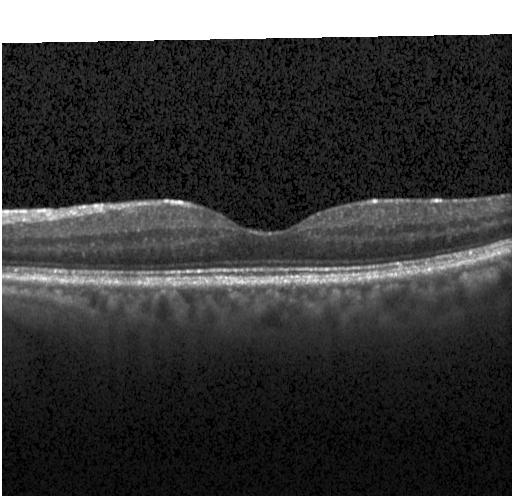 Optical coherence tomography scan; instrument: Heidelberg Spectralis. The scan shows no evidence of choroidal neovascularization, diabetic macular edema, or drusen.